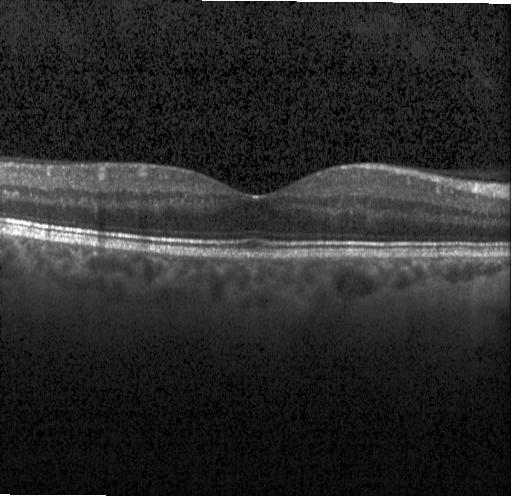 Retinal OCT cross-section showing no evidence of CNV, DME, or drusen.